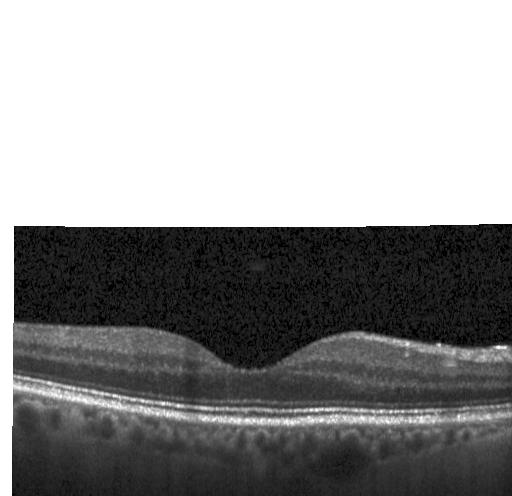

This B-scan demonstrates no CNV, no DME, and no drusen.